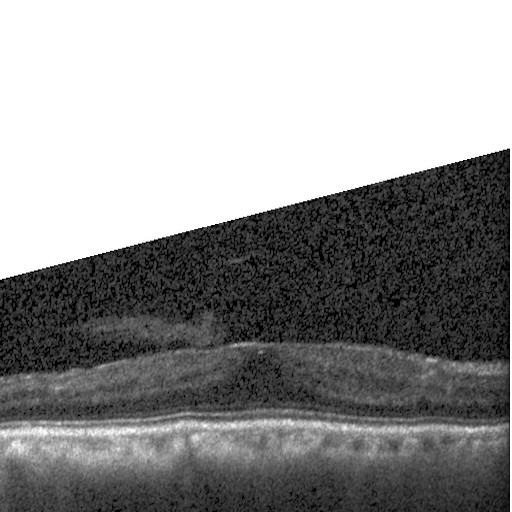 SD-OCT · macular scan · retinal OCT cross-section · Heidelberg Spectralis OCT system — OCT finding: diabetic macular edema.